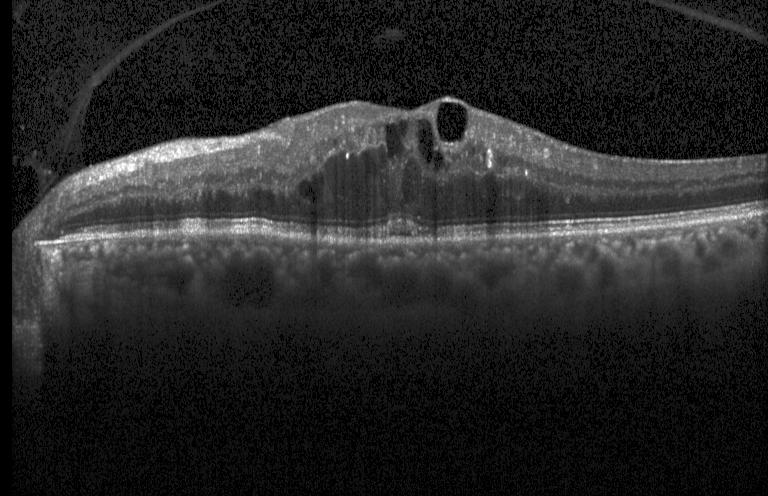 This B-scan demonstrates diabetic macular edema.